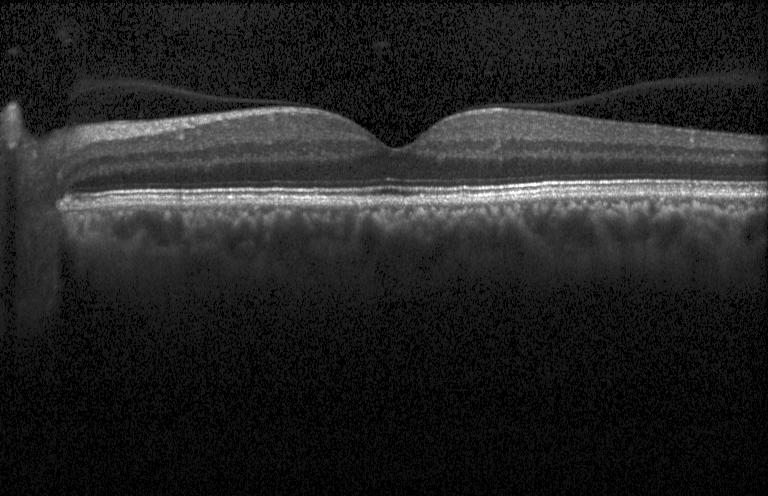

Finding: neither choroidal neovascularization, diabetic macular edema, nor drusen.